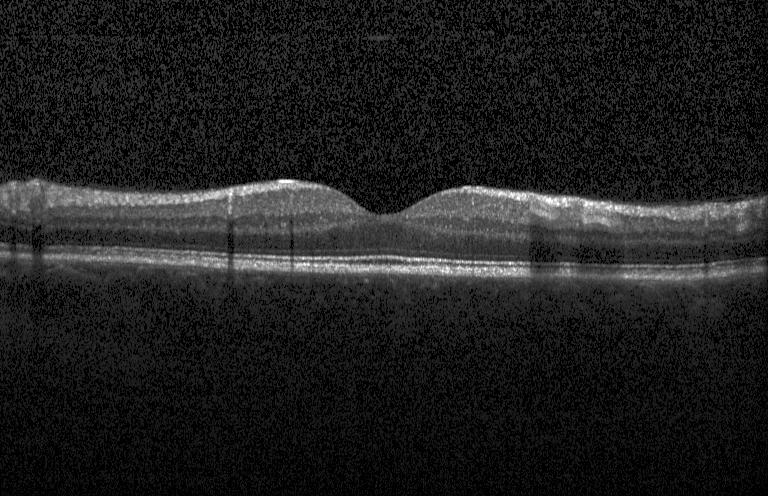 OCT scan showing no evidence of choroidal neovascularization, diabetic macular edema, or drusen.